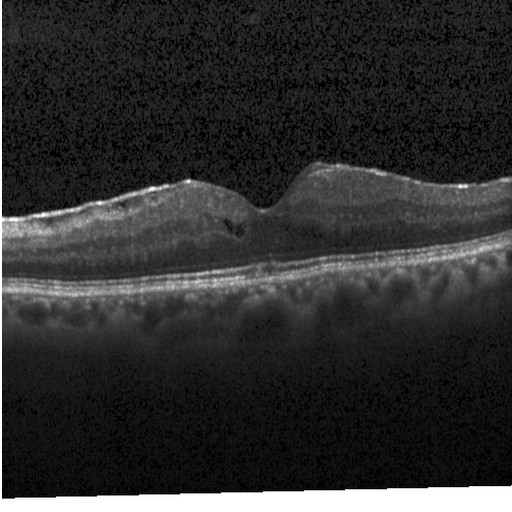 Spectral-domain optical coherence tomography · through the macula · OCT line scan. OCT finding: diabetic macular edema.